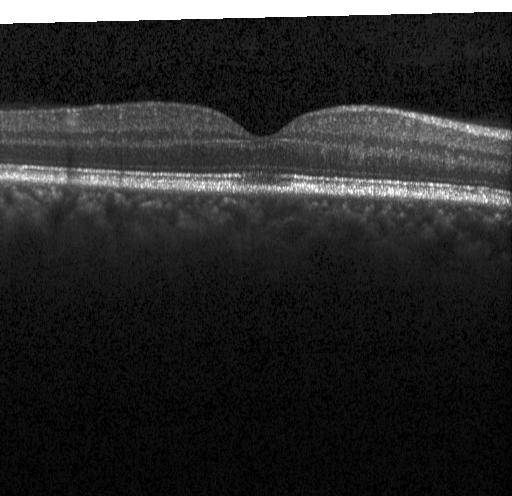

Finding: no evidence of choroidal neovascularization, diabetic macular edema, or drusen.